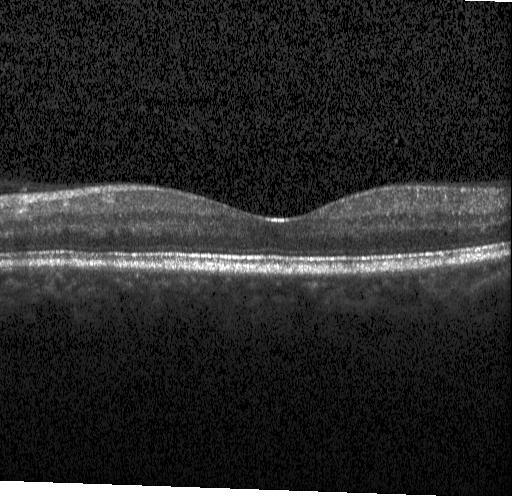

Retinal OCT B-scan. No evidence of CNV, DME, or drusen.